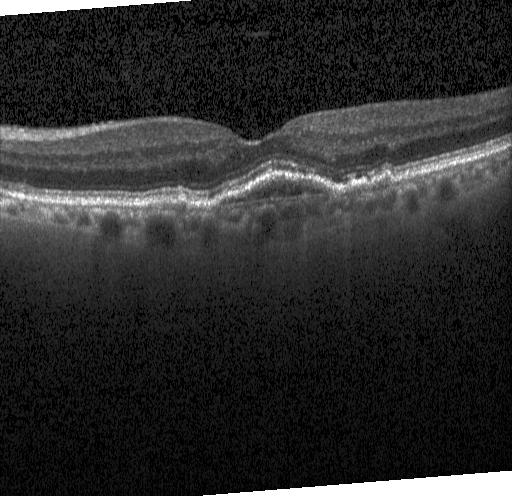
Retinal OCT cross-section — This B-scan demonstrates a choroidal neovascular membrane.